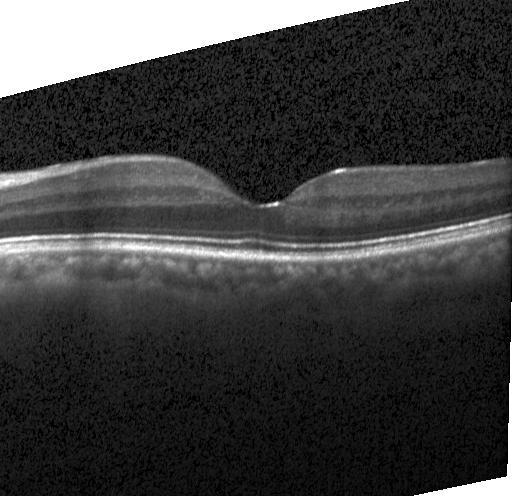 Diagnosis: no evidence of CNV, DME, or drusen.